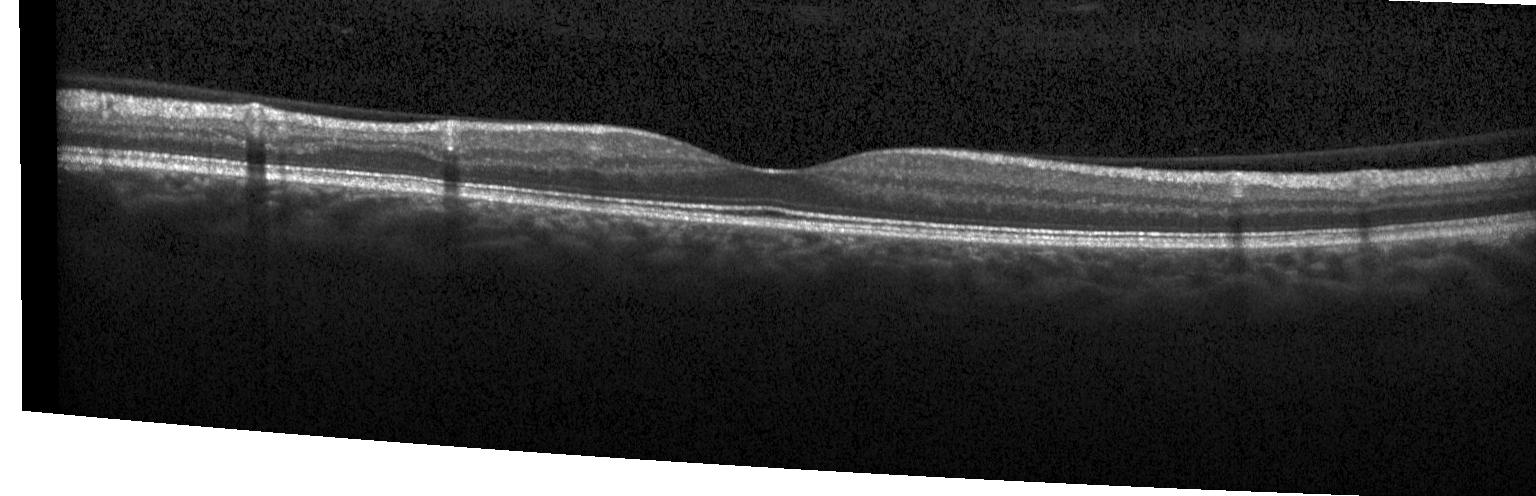
This B-scan demonstrates neither CNV, DME, nor drusen.